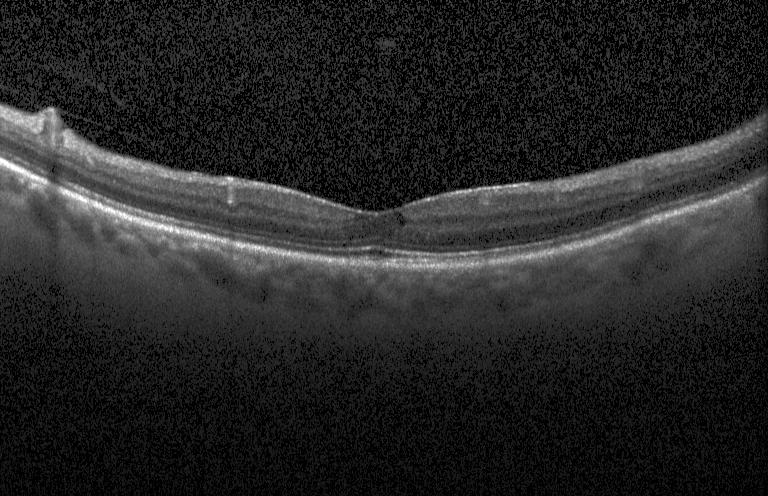 OCT B-scan · acquired on a Heidelberg Spectralis · through the macula · spectral-domain OCT.
Diagnosis: DME.